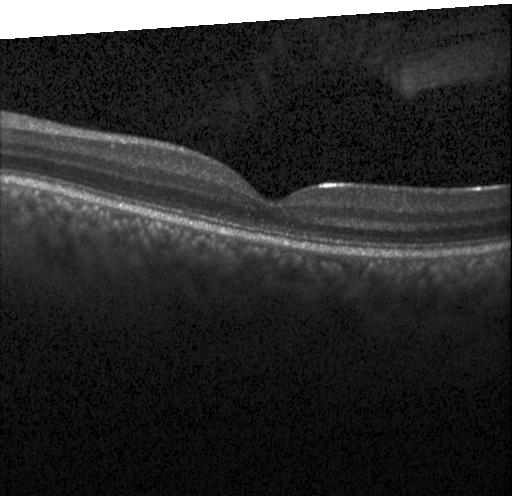

Macular scan; OCT line scan; spectral-domain OCT; instrument: Heidelberg Spectralis. Macular OCT: no choroidal neovascularization, diabetic macular edema, or drusen.